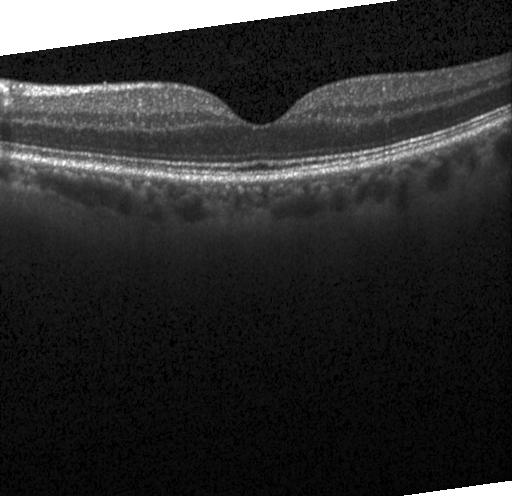
Diagnosis: no choroidal neovascularization, diabetic macular edema, or drusen.